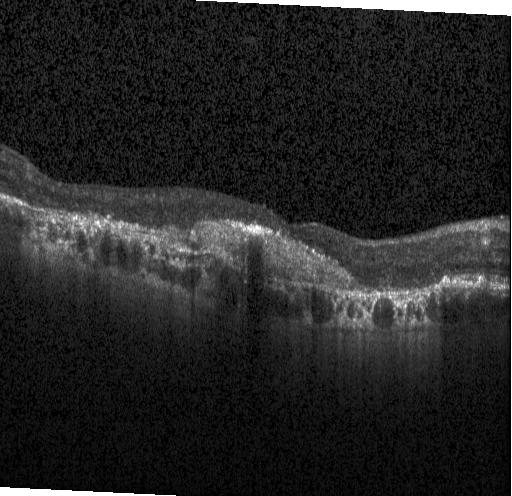

Finding: choroidal neovascularization (CNV).